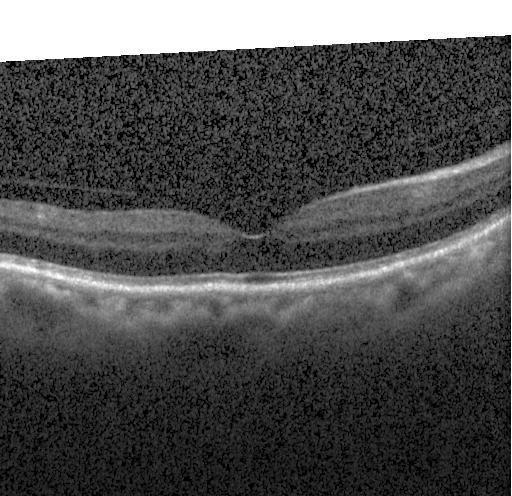 Retinal OCT cross-section showing neither choroidal neovascularization, diabetic macular edema, nor drusen.